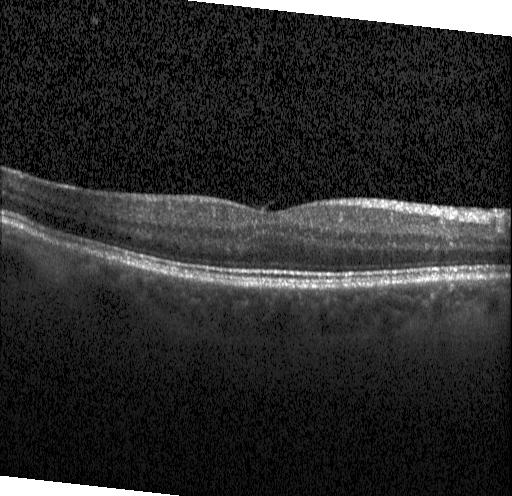
OCT B-scan showing no CNV, no DME, and no drusen.